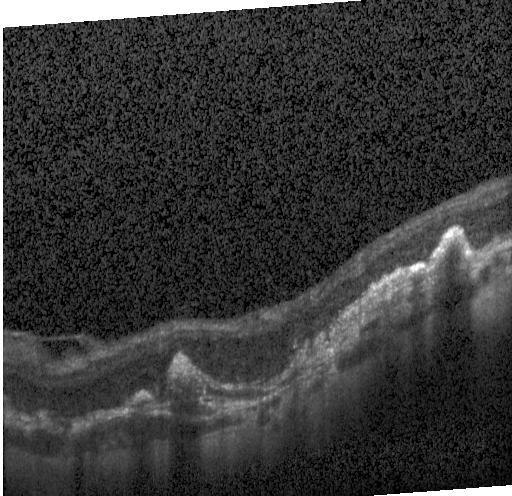 OCT finding: choroidal neovascularization.